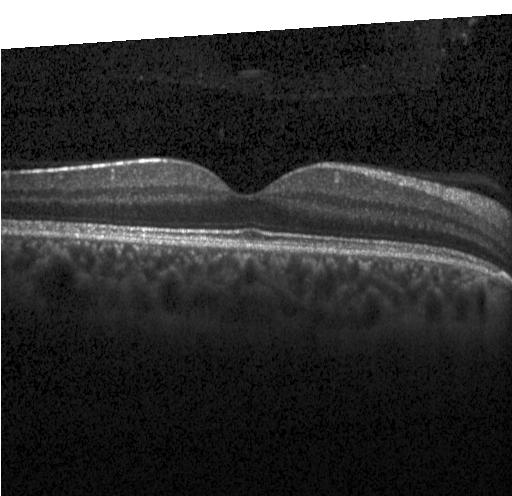
Acquired on a Heidelberg Spectralis; spectral-domain optical coherence tomography; fovea-centered; OCT B-scan — This B-scan demonstrates no CNV, no DME, and no drusen.